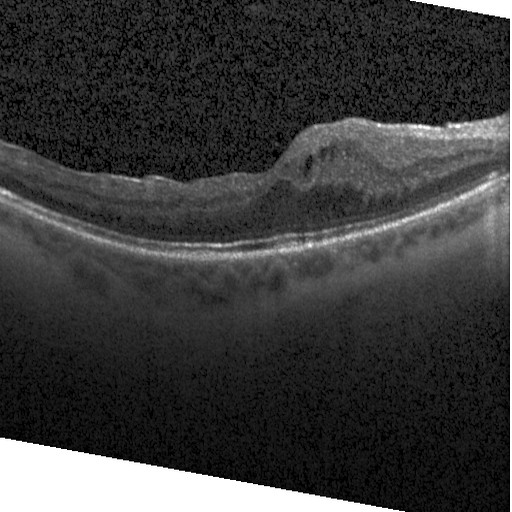
Macular scan · instrument: Heidelberg Spectralis · spectral-domain optical coherence tomography · optical coherence tomography B-scan.
Assessment: DME.